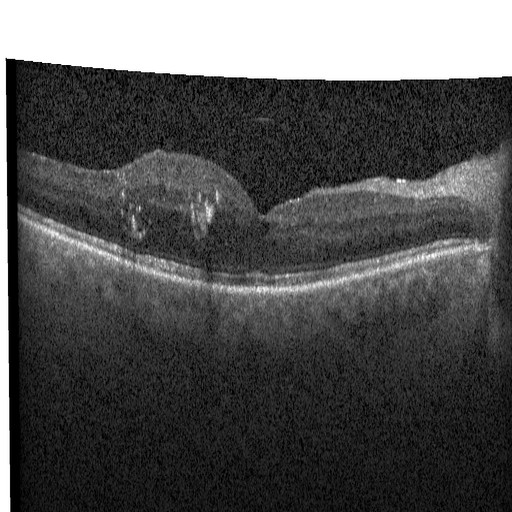
Impression: DME.